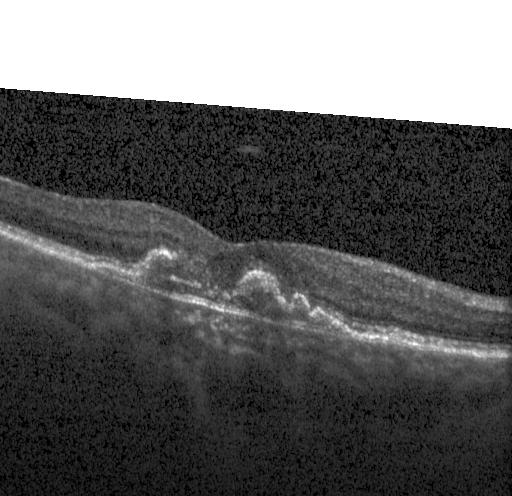

Heidelberg Spectralis; spectral-domain optical coherence tomography; through the macula; retinal OCT cross-section
This B-scan demonstrates CNV.